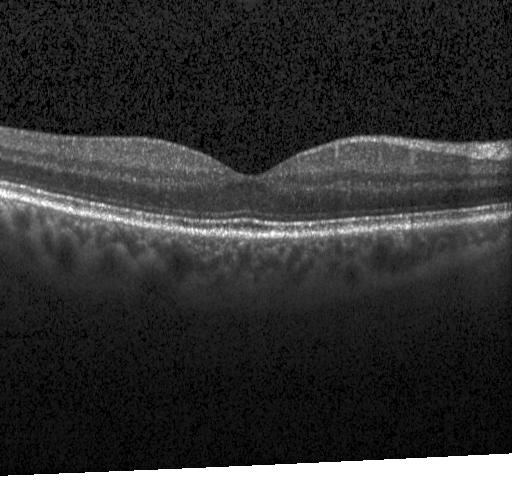
Centered on the fovea, optical coherence tomography B-scan.
No evidence of choroidal neovascularization, diabetic macular edema, or drusen.